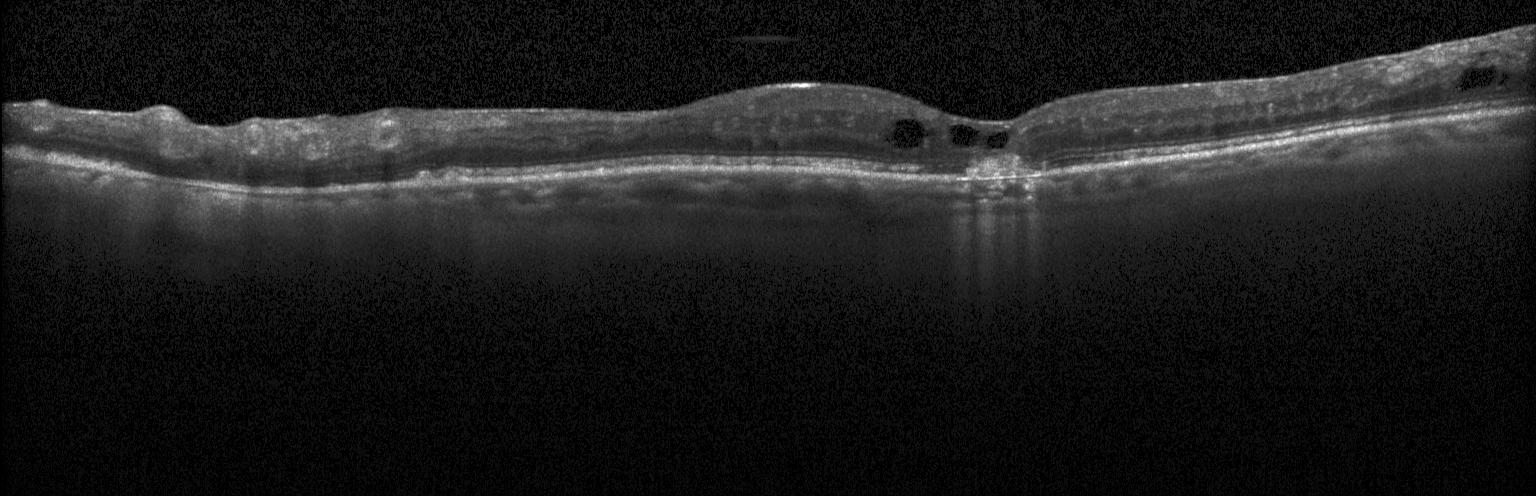

OCT B-scan, spectral-domain optical coherence tomography — Macular OCT: CNV.